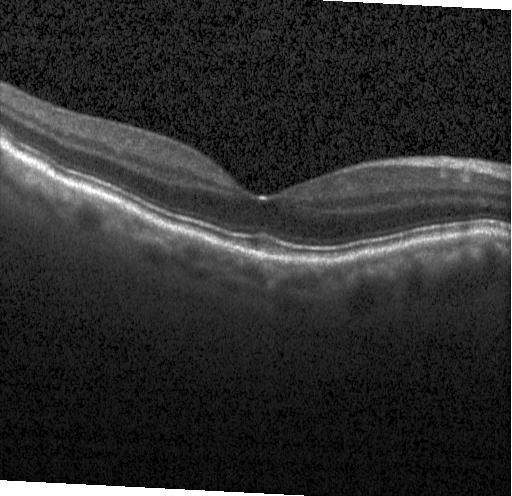

The scan shows neither choroidal neovascularization, diabetic macular edema, nor drusen.